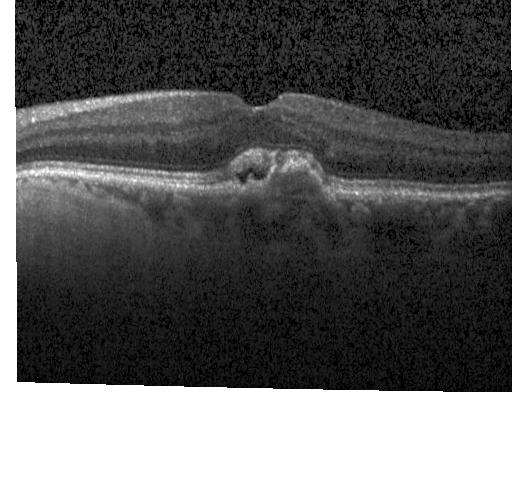
OCT finding: a choroidal neovascular membrane.